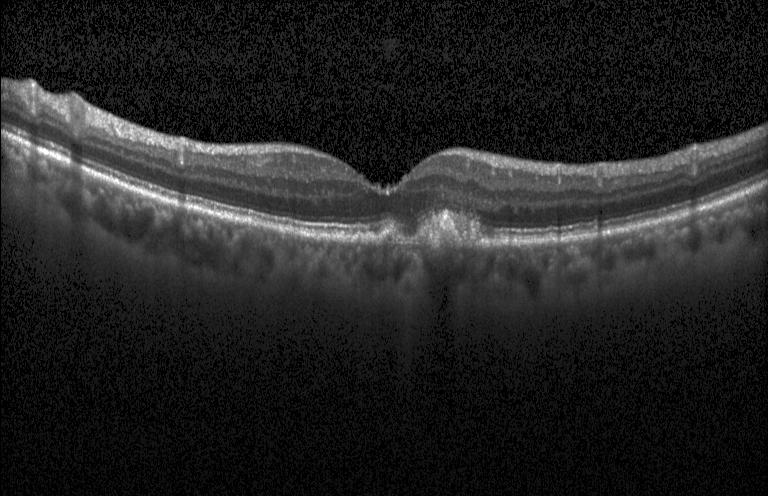 Heidelberg Spectralis OCT system; horizontal scan through the fovea; retinal OCT cross-section — Assessment: sub-RPE drusenoid deposits.